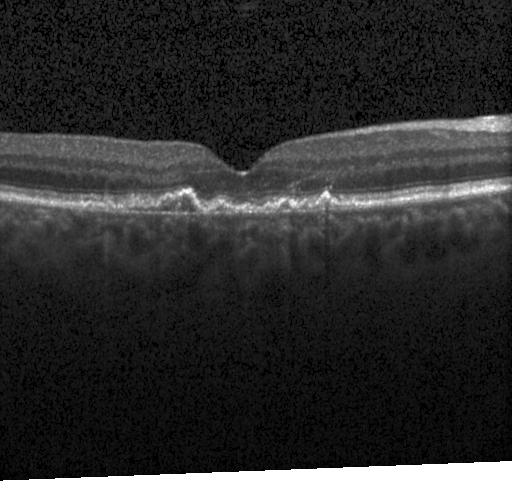

Macular OCT demonstrating CNV.